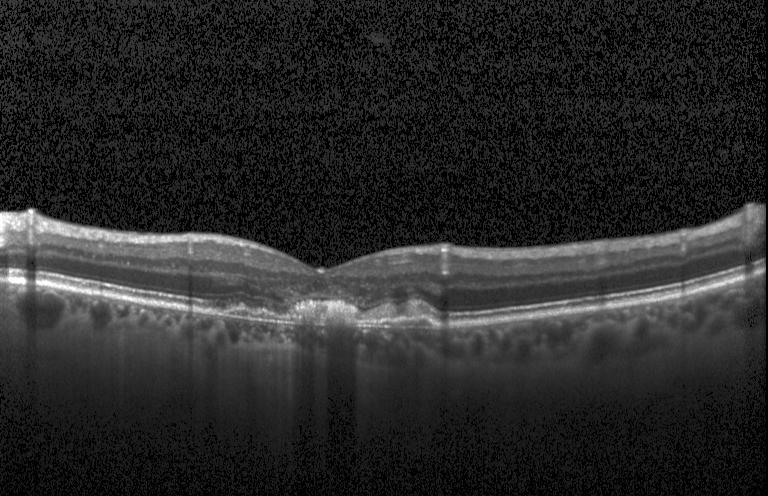

Spectral-domain OCT. Optical coherence tomography scan — CNV.